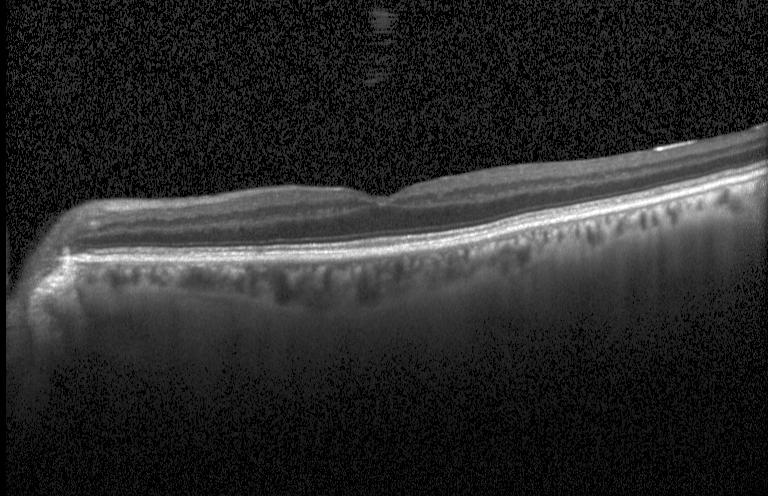 Spectral-domain OCT; fovea-centered; optical coherence tomography scan
This B-scan demonstrates neither choroidal neovascularization, diabetic macular edema, nor drusen.